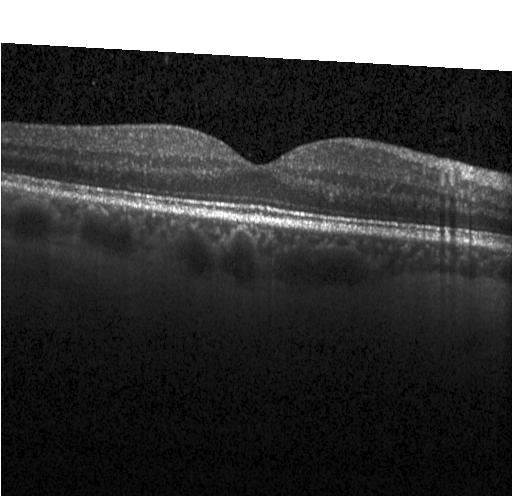

Macular OCT demonstrating no choroidal neovascularization, diabetic macular edema, or drusen.